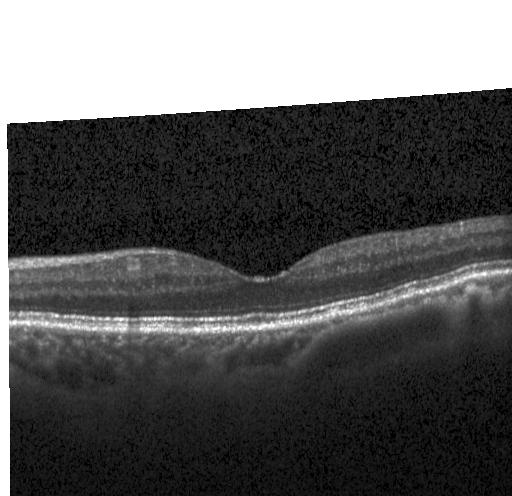
Horizontal scan through the fovea · Heidelberg Spectralis · optical coherence tomography scan.
This B-scan demonstrates no choroidal neovascularization, diabetic macular edema, or drusen.